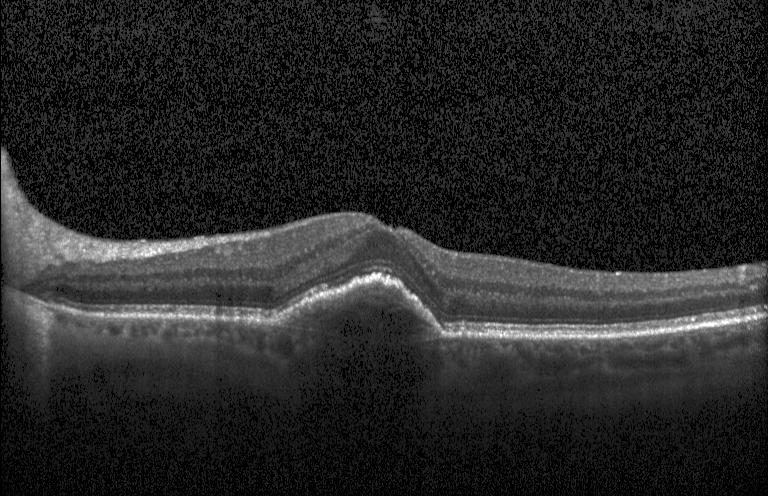
OCT B-scan showing a choroidal neovascular membrane.